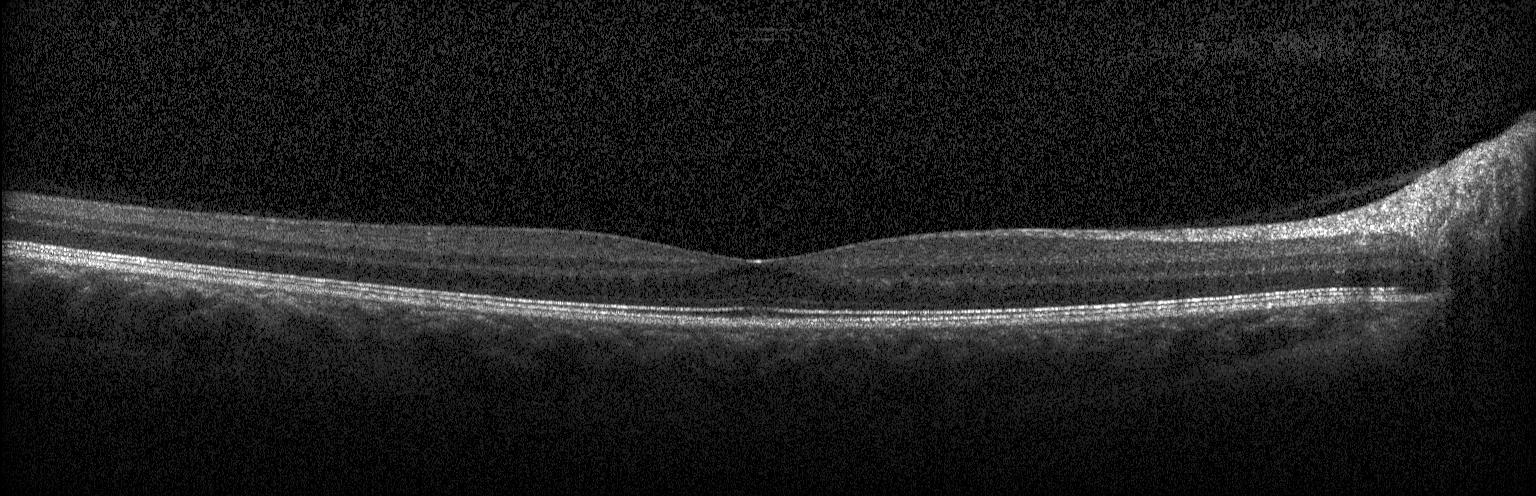 Macular OCT: no choroidal neovascularization, no diabetic macular edema, and no drusen.